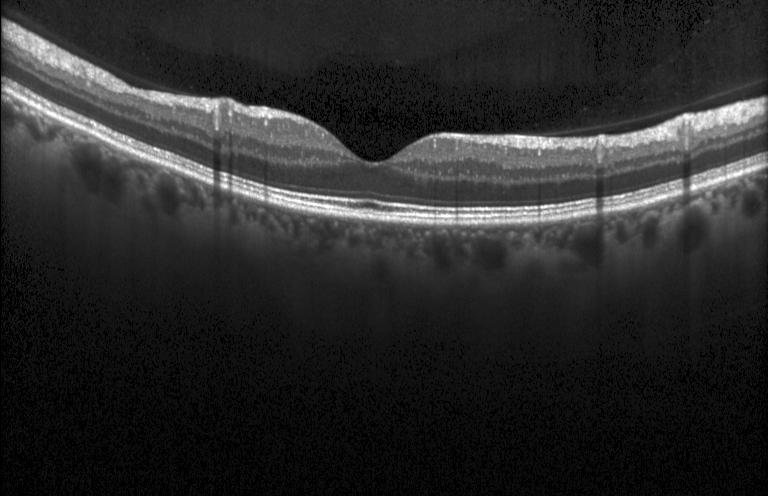
Diagnosis: no CNV, no DME, and no drusen.